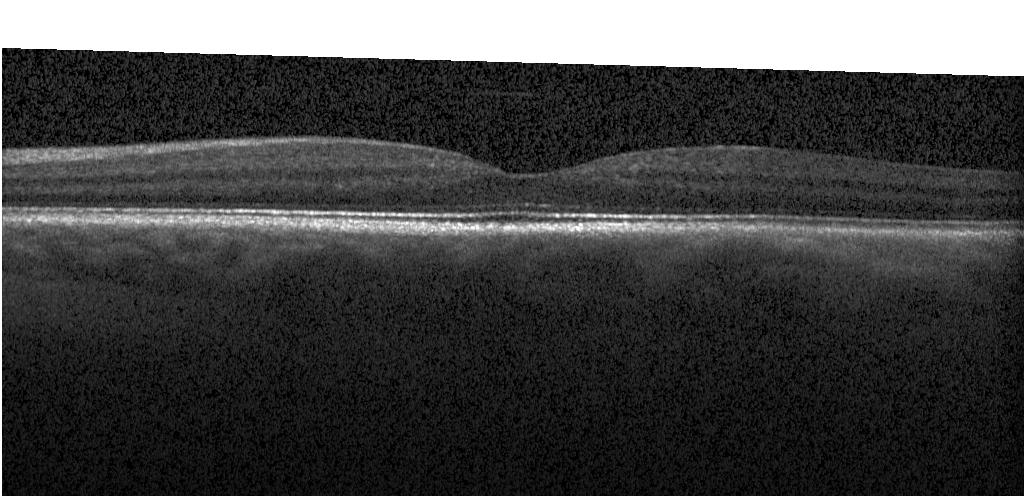 Spectral-domain optical coherence tomography; OCT line scan. Diagnosis: neither CNV, DME, nor drusen.